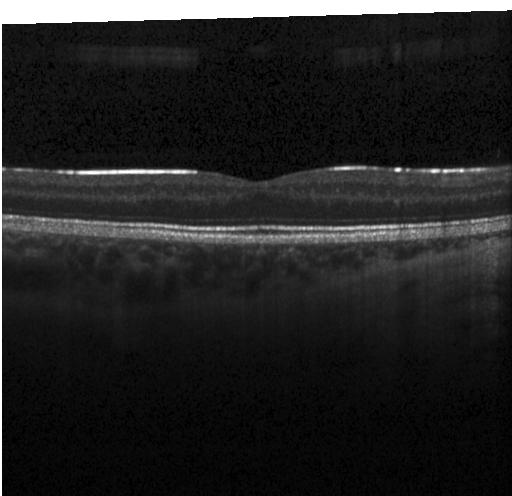 Fovea-centered. Optical coherence tomography scan. Spectral-domain OCT. Acquired on a Heidelberg Spectralis
The scan shows no choroidal neovascularization, diabetic macular edema, or drusen.